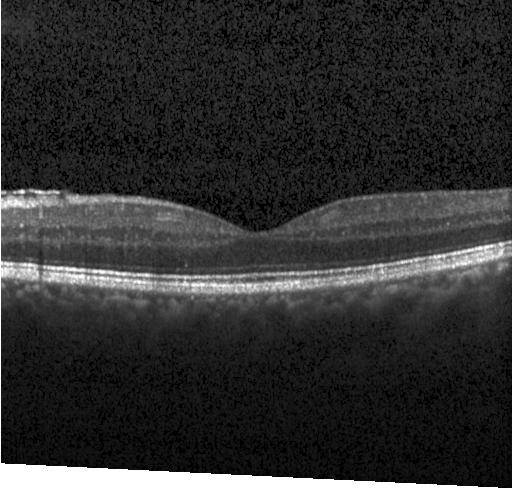 Retinal OCT cross-section.
Dx: no CNV, no DME, and no drusen.